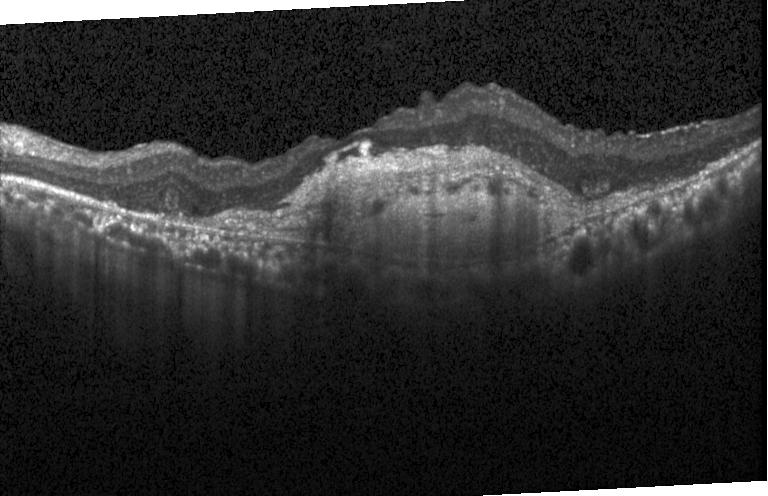

Finding: choroidal neovascularization.